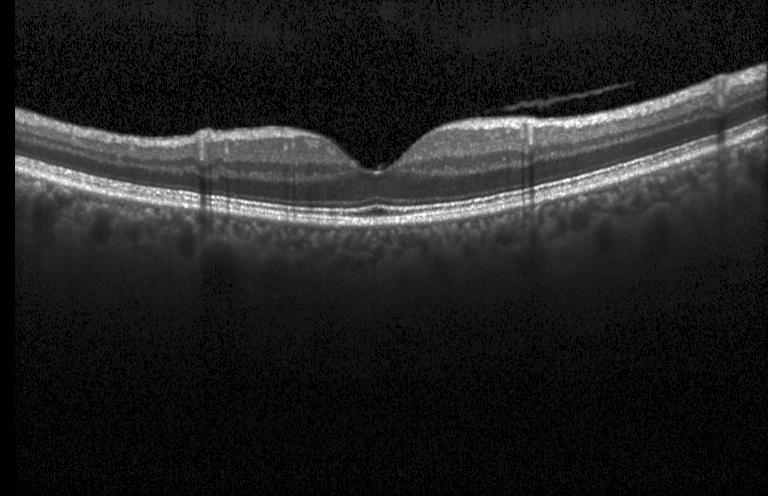 Retinal OCT cross-section, SD-OCT, acquired on a Heidelberg Spectralis. Impression: no evidence of choroidal neovascularization, diabetic macular edema, or drusen.